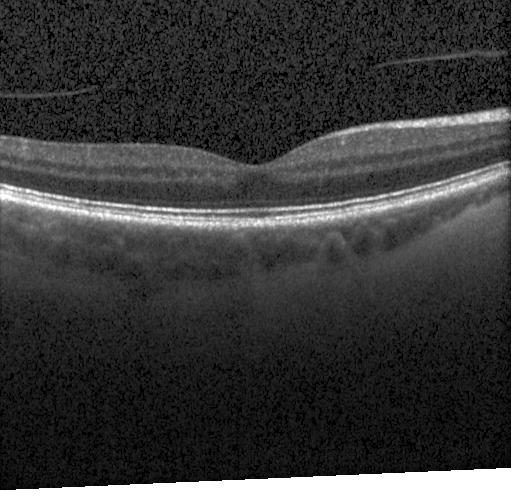
OCT B-scan
No evidence of choroidal neovascularization, diabetic macular edema, or drusen.